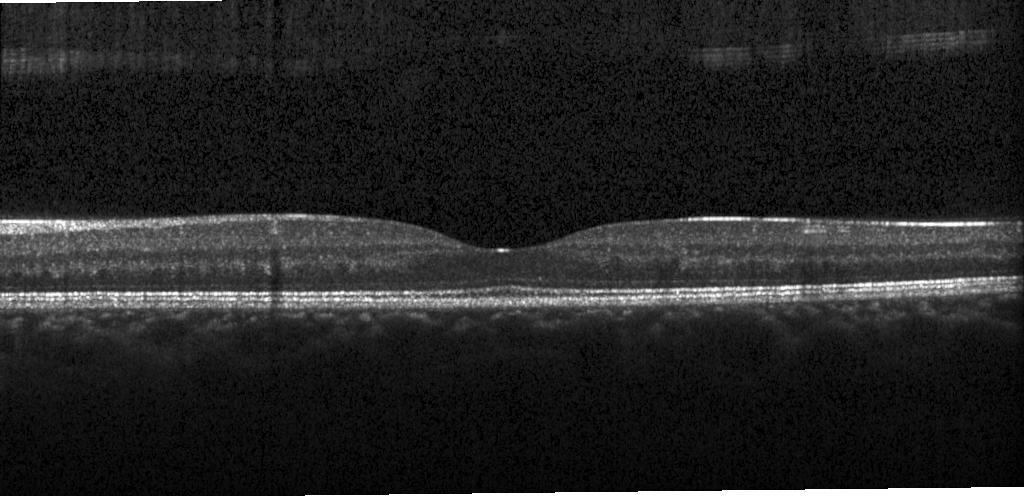 OCT finding: neither choroidal neovascularization, diabetic macular edema, nor drusen.